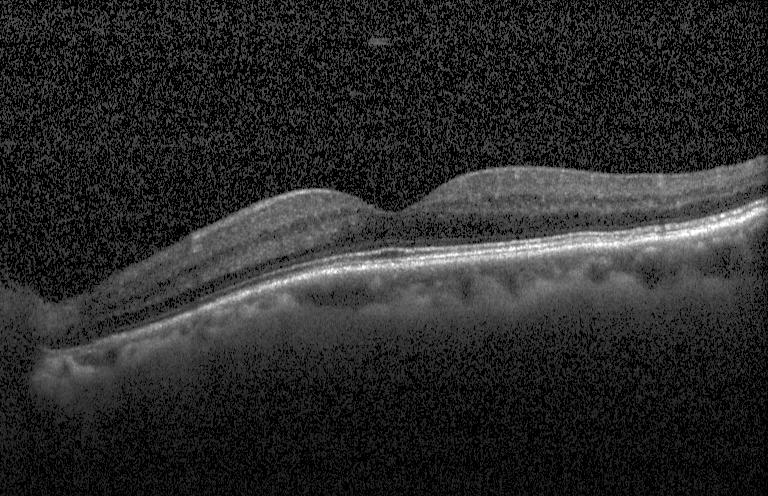
Retinal OCT cross-section
Diagnosis: no choroidal neovascularization, no diabetic macular edema, and no drusen.